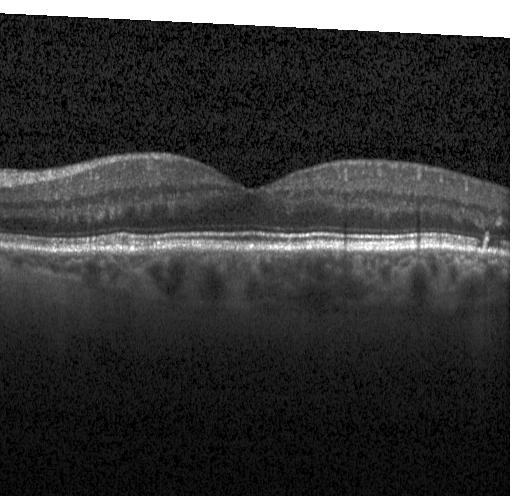 OCT line scan; spectral-domain OCT; macular scan; acquired on a Heidelberg Spectralis
Assessment: no CNV, no DME, and no drusen.